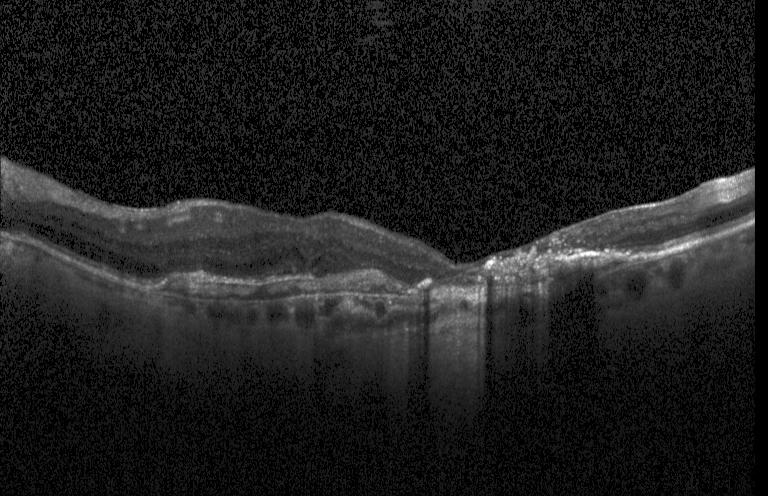
Finding: CNV.